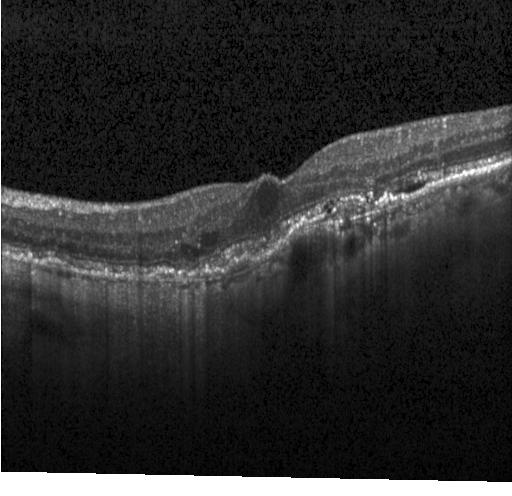
SD-OCT, centered on the fovea, instrument: Heidelberg Spectralis, OCT line scan
Finding: choroidal neovascularization (CNV).